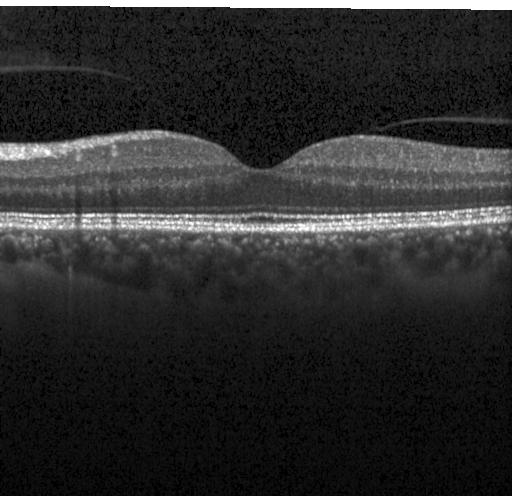
Diagnosis: no CNV, DME, or drusen.